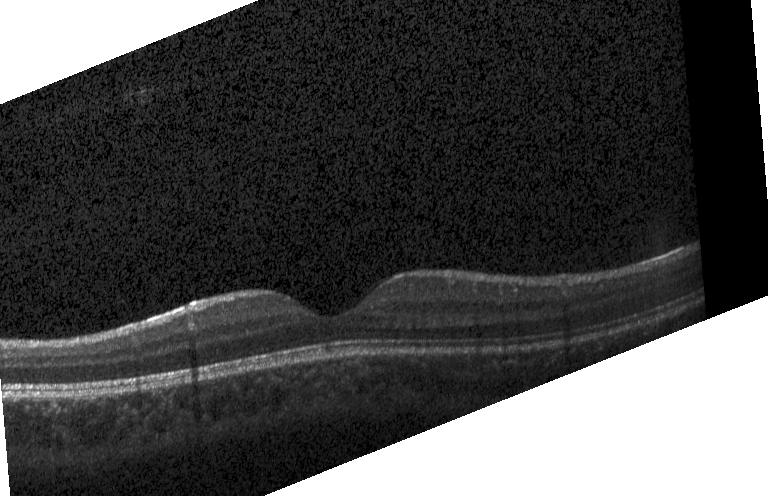
OCT finding: no evidence of choroidal neovascularization, diabetic macular edema, or drusen.